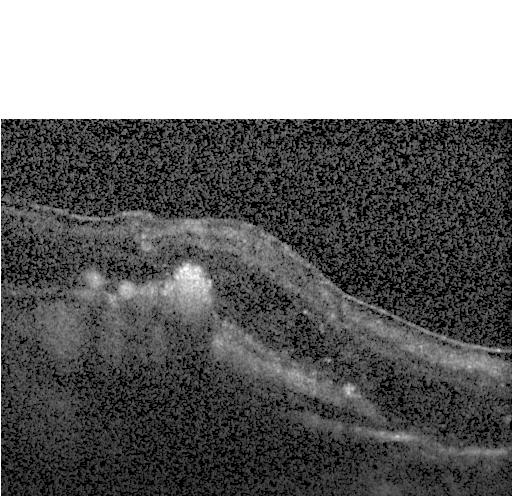

Dx: choroidal neovascularization.